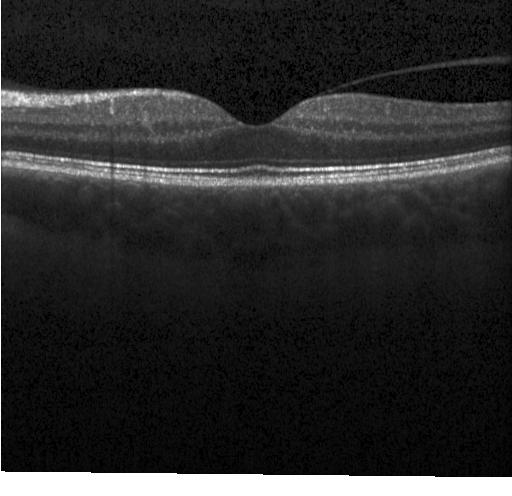
Impression: no choroidal neovascularization, diabetic macular edema, or drusen.